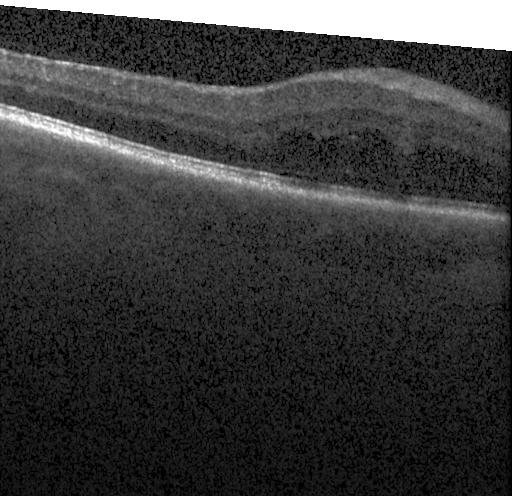 Horizontal scan through the fovea; OCT B-scan.
Macular OCT: diabetic macular edema.